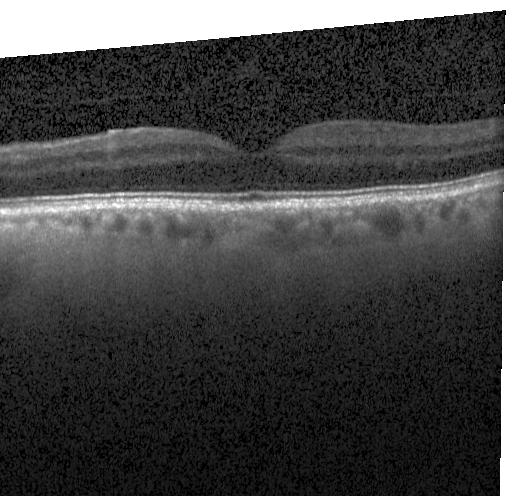
OCT finding: no choroidal neovascularization, diabetic macular edema, or drusen.